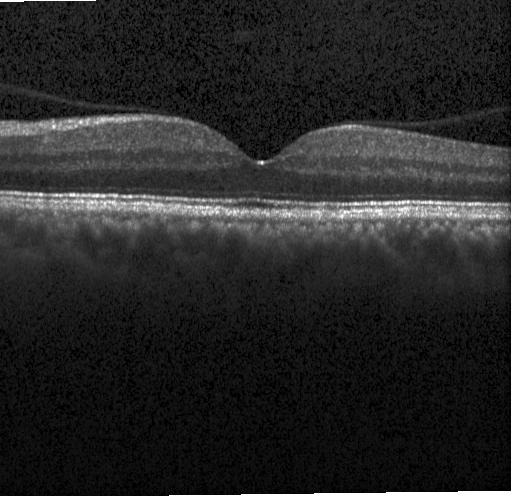
Spectral-domain OCT, instrument: Heidelberg Spectralis, OCT B-scan. Neither choroidal neovascularization, diabetic macular edema, nor drusen.